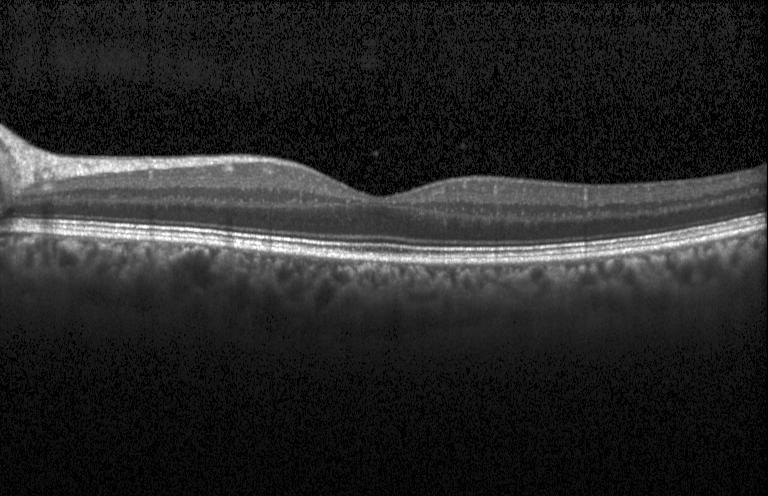

Optical coherence tomography scan, Heidelberg Spectralis, through the macula, SD-OCT. Assessment: no evidence of CNV, DME, or drusen.